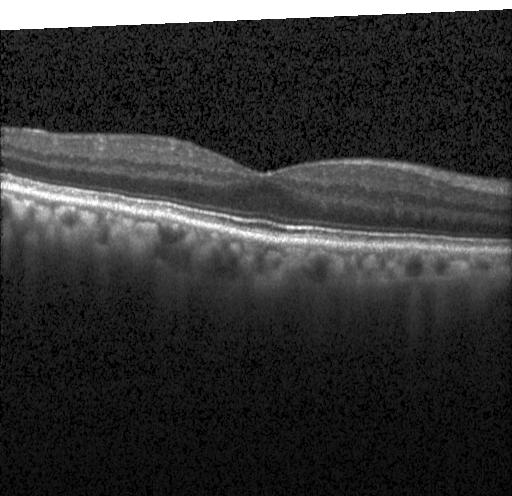
Retinal OCT cross-section, spectral-domain optical coherence tomography, acquired on a Heidelberg Spectralis, centered on the fovea
Assessment: no choroidal neovascularization, diabetic macular edema, or drusen.